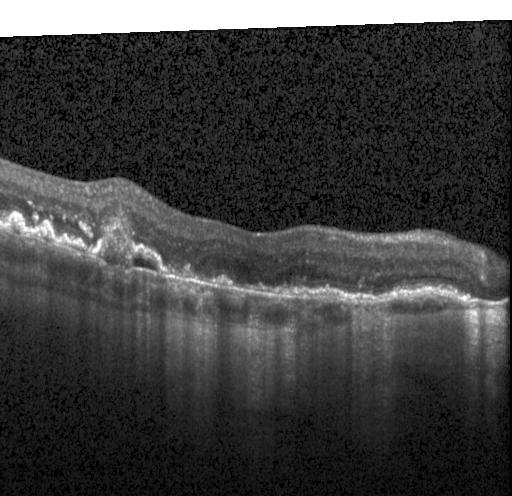

Optical coherence tomography B-scan, spectral-domain optical coherence tomography
Finding: a choroidal neovascular membrane.